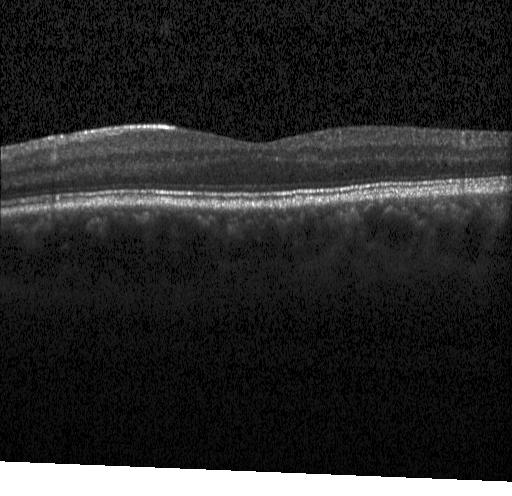

Centered on the fovea, OCT line scan — Diagnosis: no choroidal neovascularization, diabetic macular edema, or drusen.